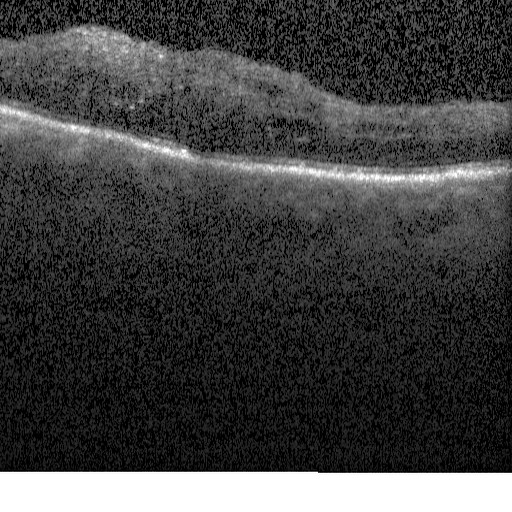 Dx: diabetic macular edema.